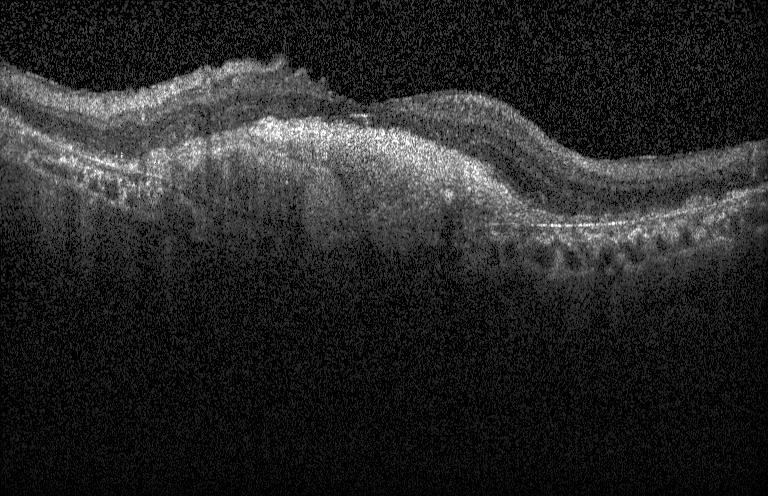
Choroidal neovascularization (CNV).